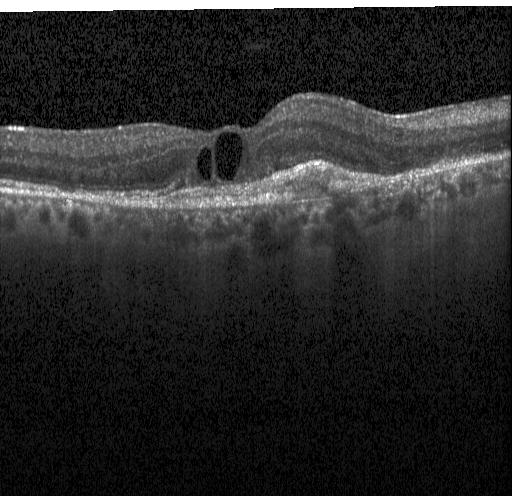

SD-OCT · Heidelberg Spectralis · OCT B-scan — Macular OCT: CNV.